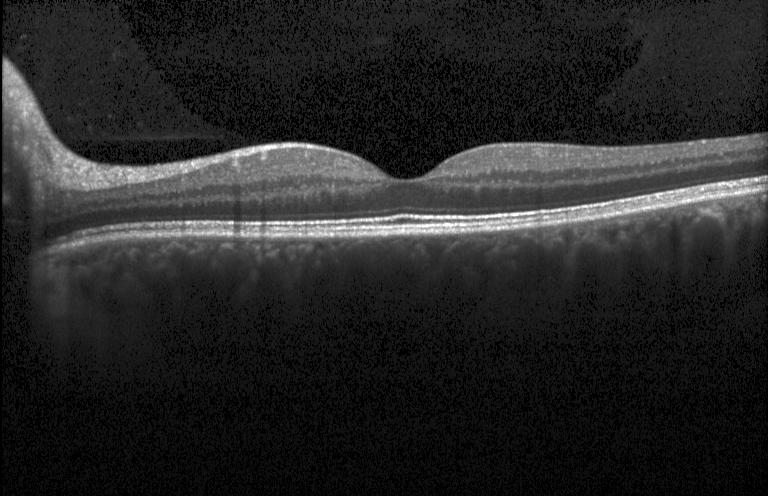

Optical coherence tomography B-scan · fovea-centered · spectral-domain optical coherence tomography
This B-scan demonstrates no choroidal neovascularization, diabetic macular edema, or drusen.